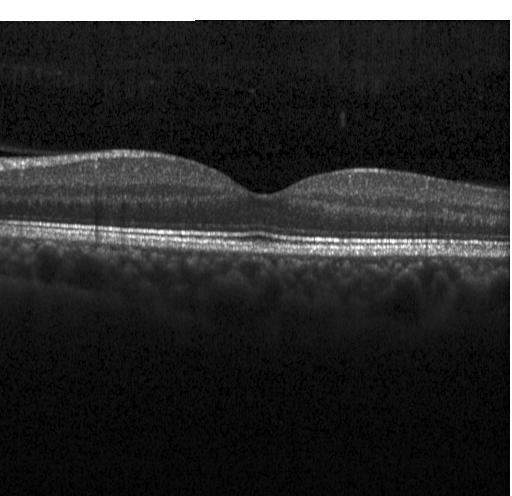
Finding: no evidence of choroidal neovascularization, diabetic macular edema, or drusen.